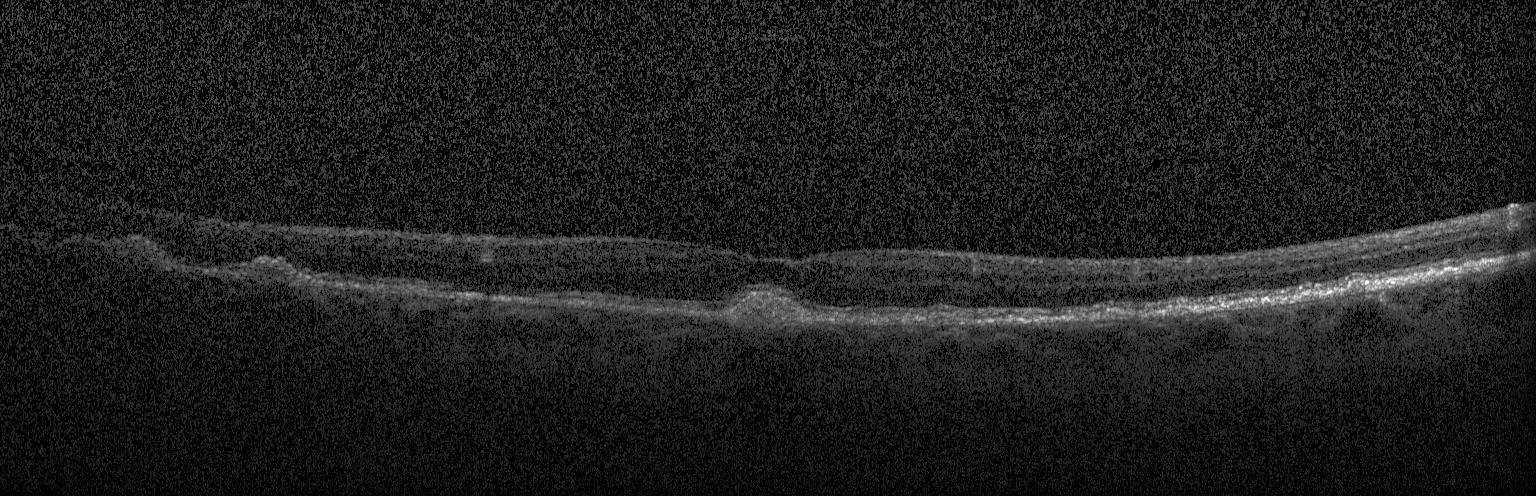 Retinal OCT cross-section showing sub-RPE drusenoid deposits.